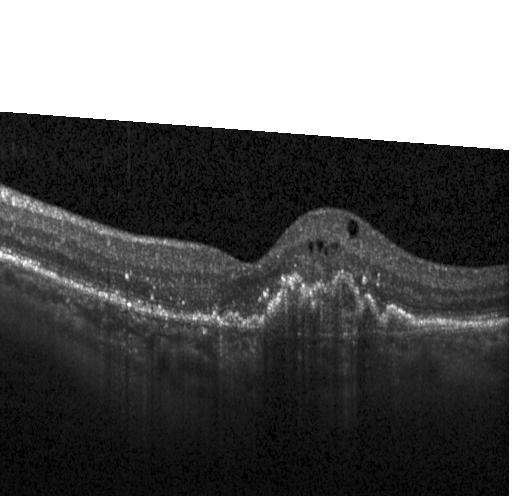
OCT B-scan
Finding: choroidal neovascularization.